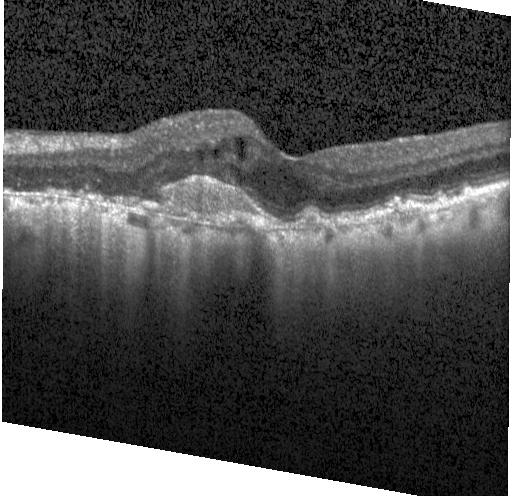 Optical coherence tomography scan. This B-scan demonstrates a choroidal neovascular membrane.